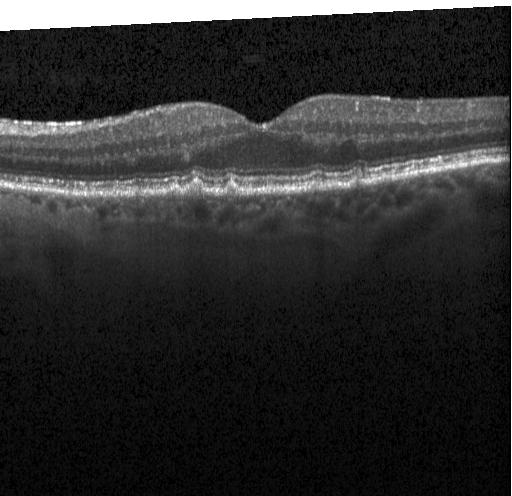

Diagnosis: sub-RPE drusenoid deposits.